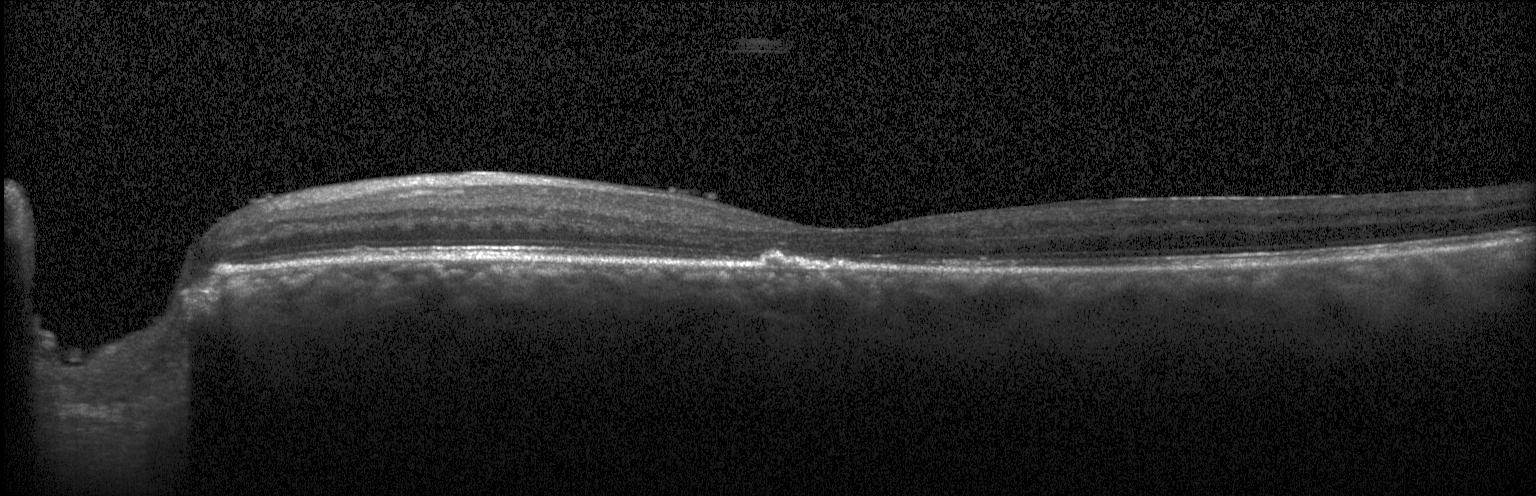
OCT line scan. Horizontal scan through the fovea. SD-OCT
Diagnosis: multiple drusen.